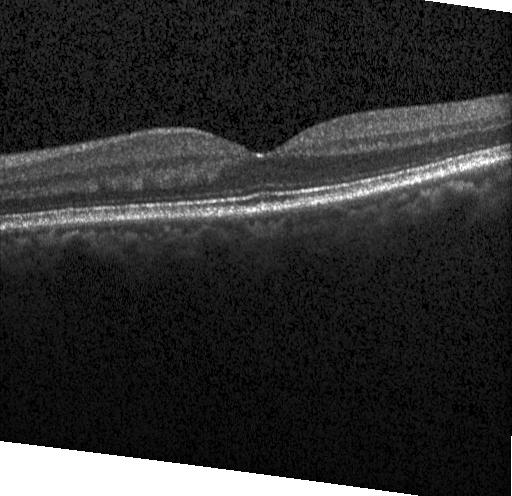

Heidelberg Spectralis · optical coherence tomography scan · fovea-centered.
Macular OCT: no CNV, DME, or drusen.